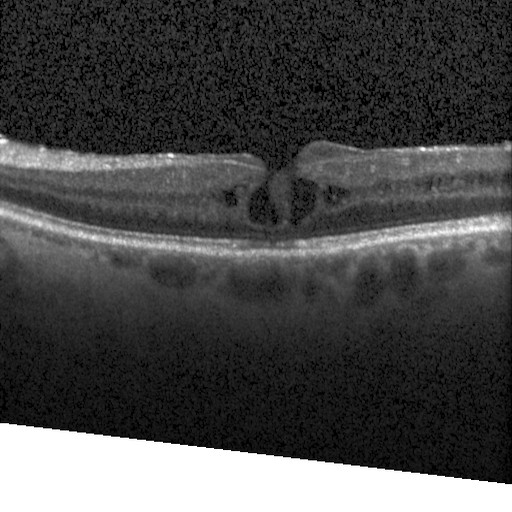
Retinal OCT cross-section showing DME.